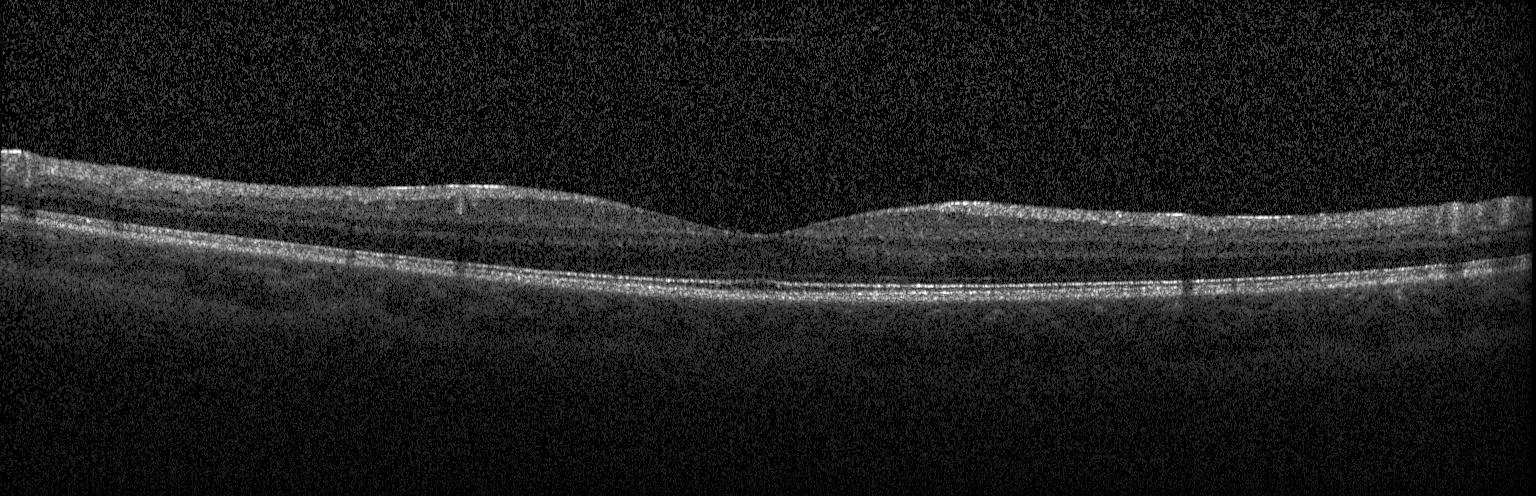 Finding: no CNV, no DME, and no drusen.